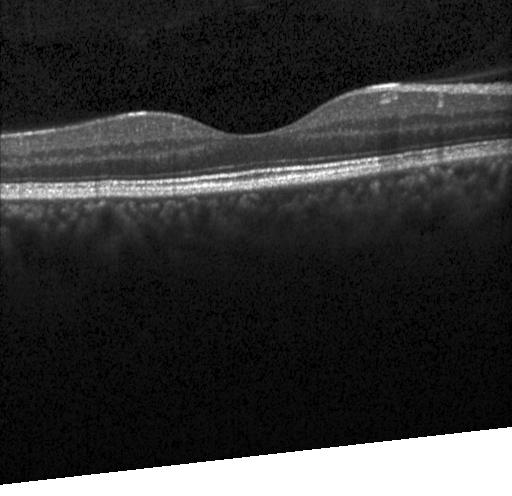
OCT B-scan showing no choroidal neovascularization, no diabetic macular edema, and no drusen.